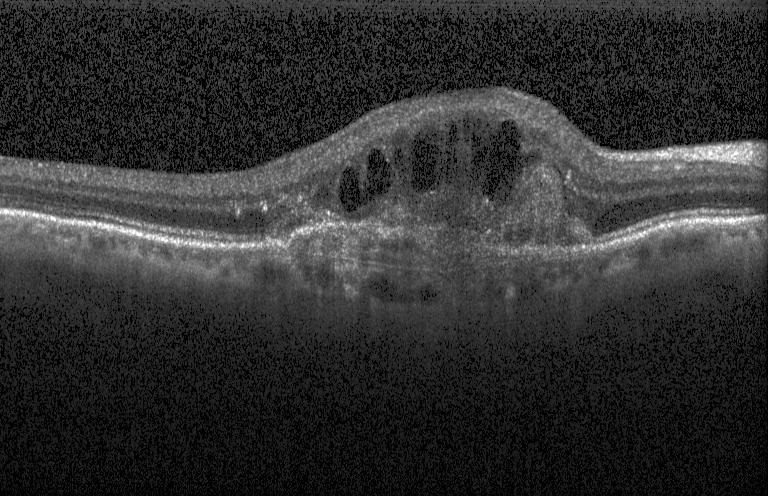

Optical coherence tomography scan — A choroidal neovascular membrane.